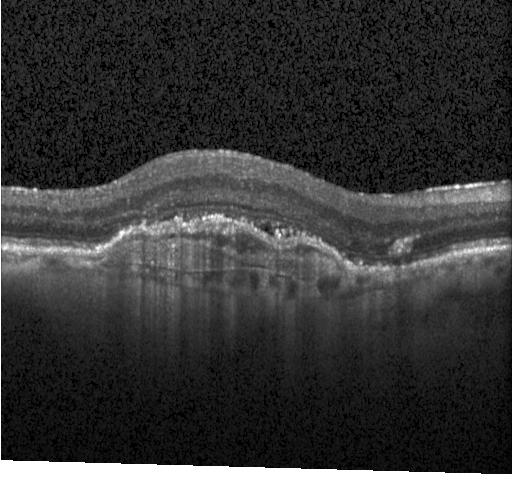

Spectral-domain optical coherence tomography; fovea-centered; Heidelberg Spectralis; retinal OCT B-scan.
This B-scan demonstrates a choroidal neovascular membrane.